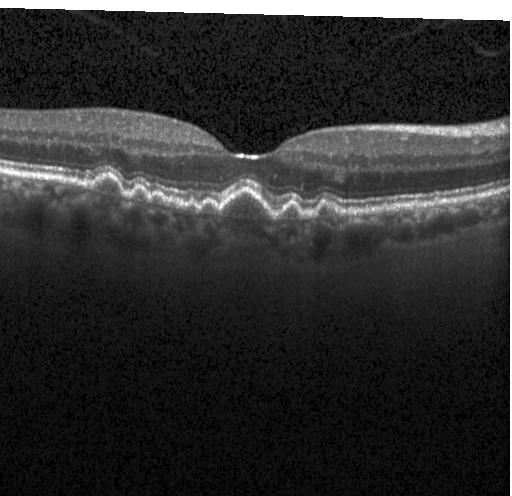
Acquired on a Heidelberg Spectralis · optical coherence tomography B-scan · through the macula.
Diagnosis: sub-RPE drusenoid deposits.